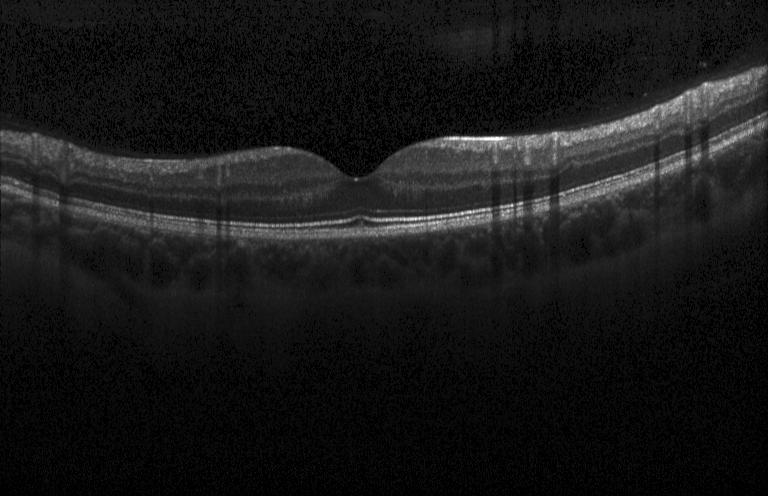
Macular OCT: neither choroidal neovascularization, diabetic macular edema, nor drusen.